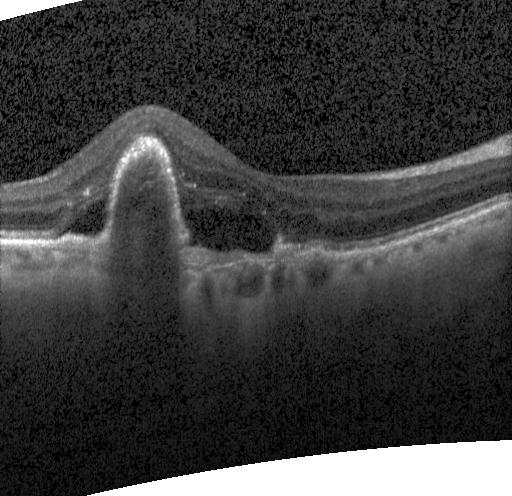 Assessment: a choroidal neovascular membrane.